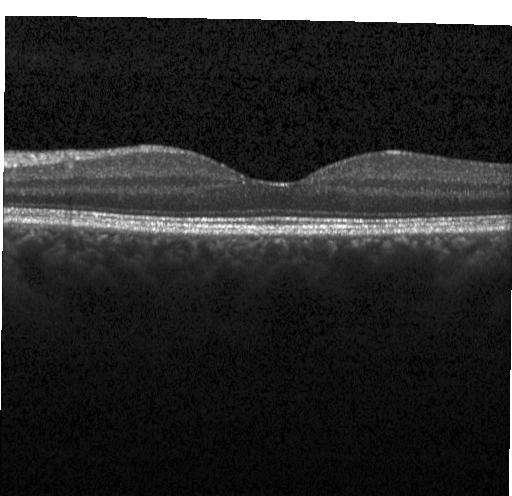
Macular scan. Optical coherence tomography B-scan — This B-scan demonstrates no CNV, DME, or drusen.